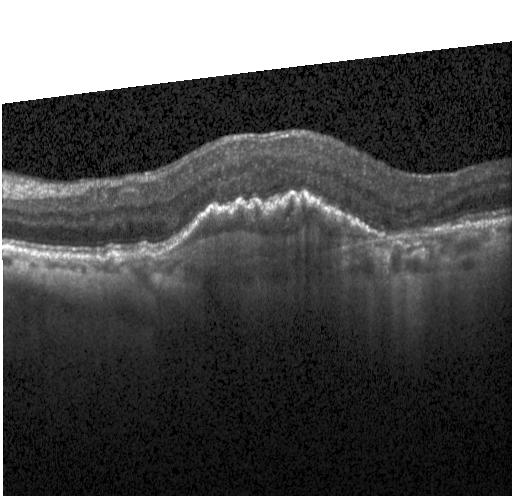
This B-scan demonstrates a choroidal neovascular membrane.